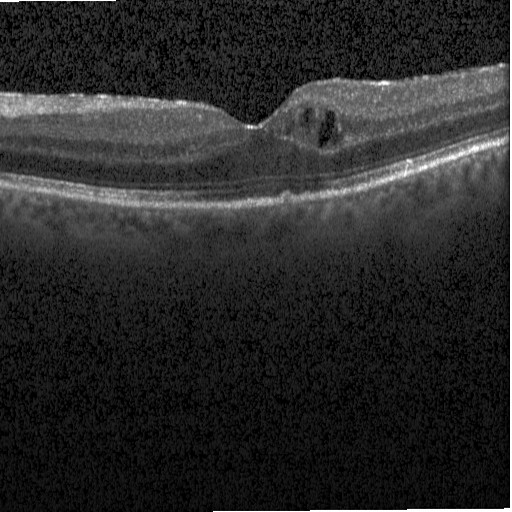

Macular OCT: diabetic macular edema.